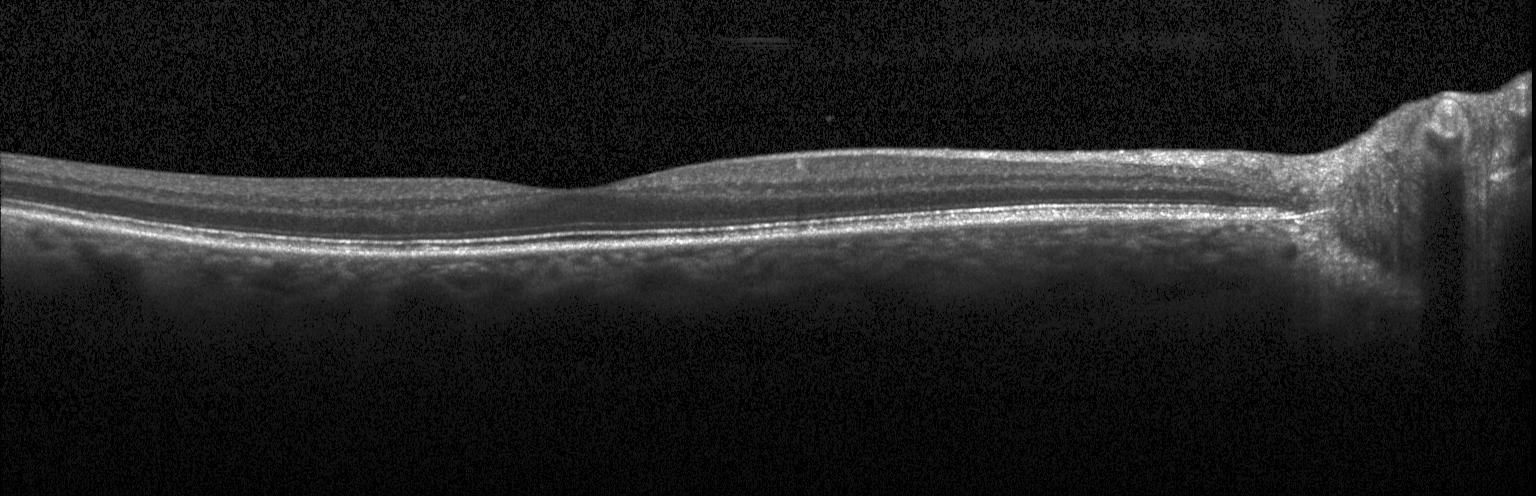
Impression: no choroidal neovascularization, no diabetic macular edema, and no drusen.